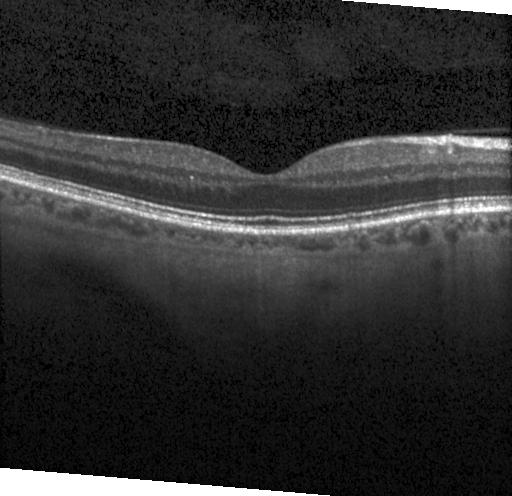

Diagnosis: neither CNV, DME, nor drusen.